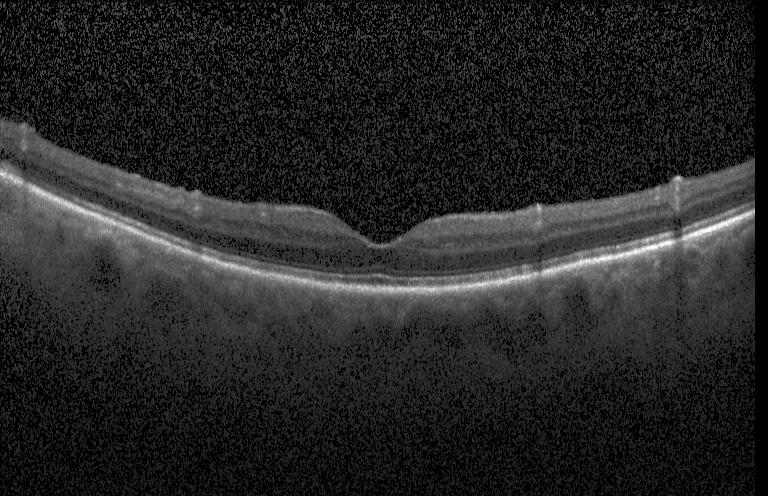 Impression: no choroidal neovascularization, no diabetic macular edema, and no drusen.